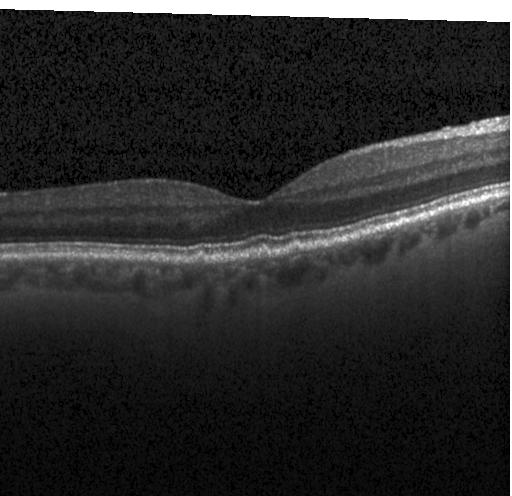
Finding: sub-RPE drusenoid deposits.